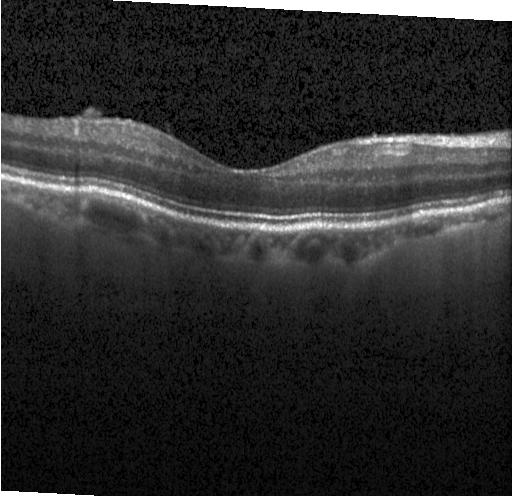

OCT finding: no choroidal neovascularization, no diabetic macular edema, and no drusen.